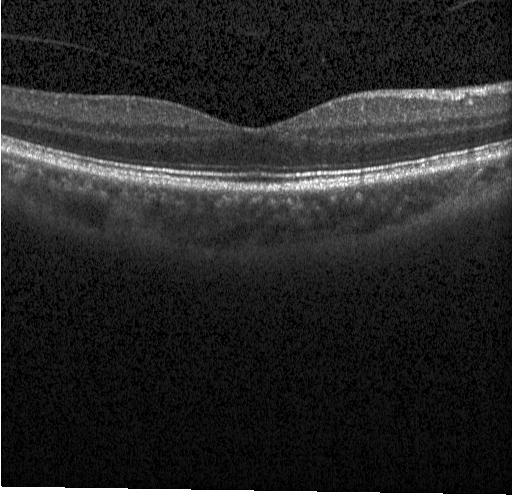
Retinal OCT cross-section, through the macula — Macular OCT: neither CNV, DME, nor drusen.